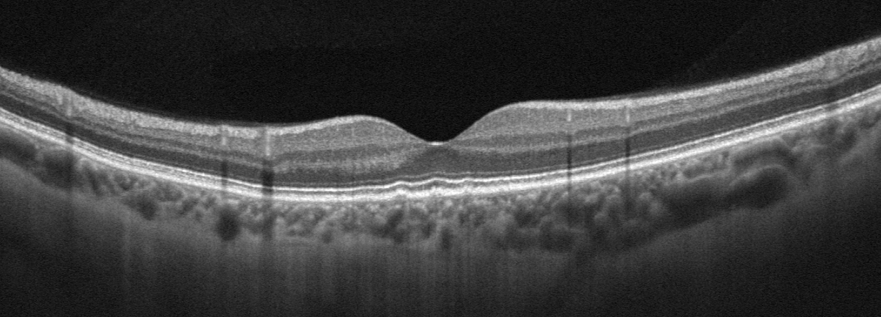
Optical coherence tomography scan; fovea-centered.
Assessment: age-related macular degeneration (AMD).